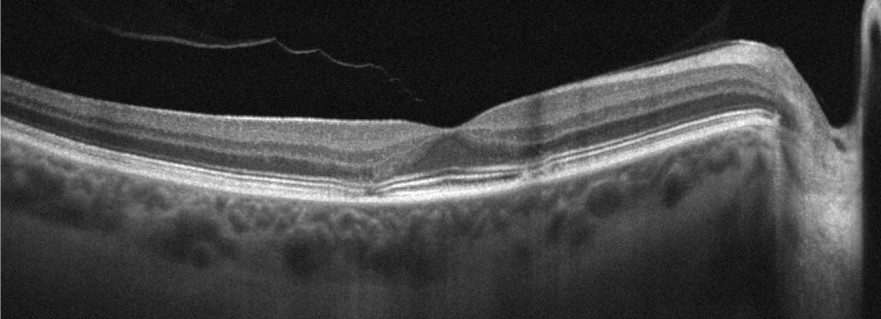 Retinal OCT B-scan · acquired on an Optovue Avanti RTVue XR. Assessment: age-related macular degeneration.